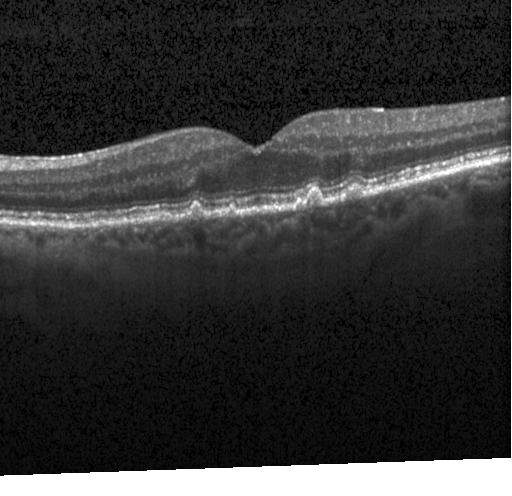
Finding: sub-RPE drusenoid deposits.